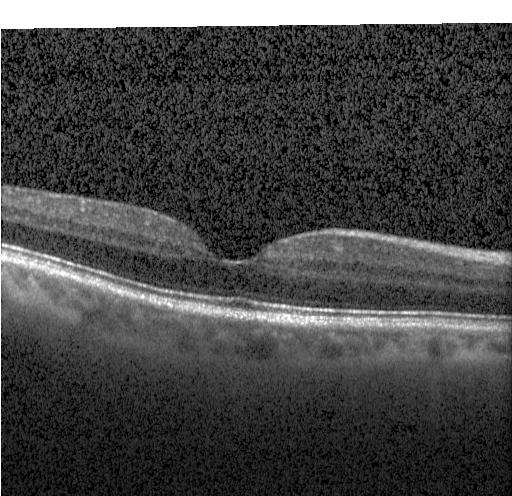
Optical coherence tomography scan, spectral-domain OCT, instrument: Heidelberg Spectralis. Diagnosis: no choroidal neovascularization, no diabetic macular edema, and no drusen.